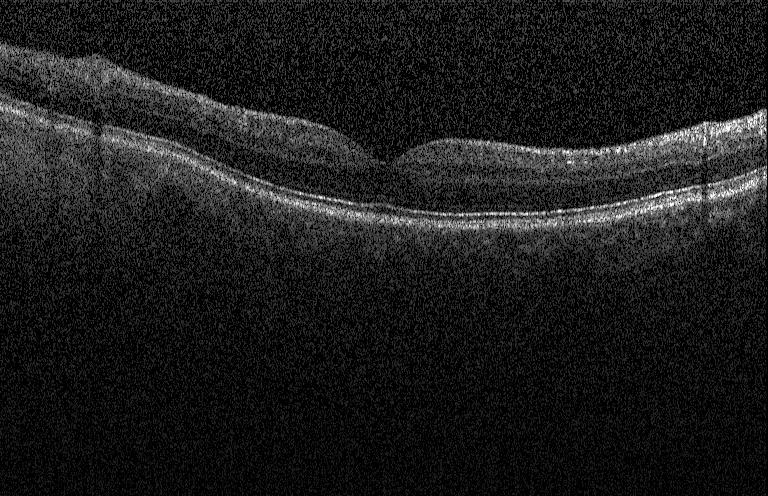

Impression: no choroidal neovascularization, diabetic macular edema, or drusen.